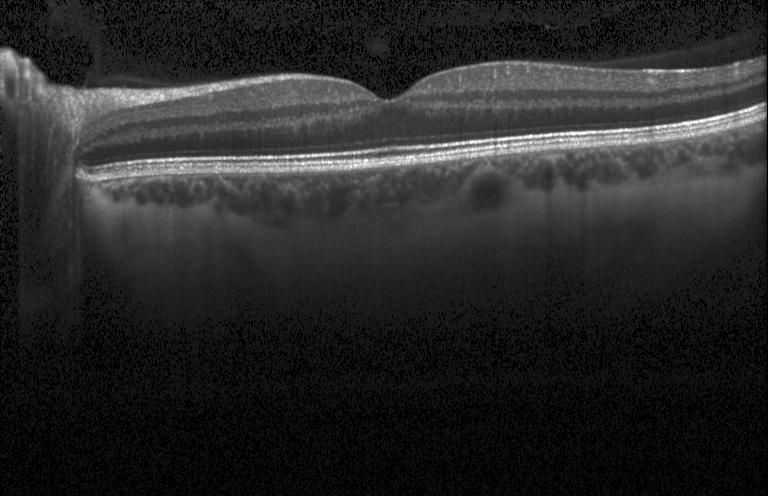 The scan shows no choroidal neovascularization, no diabetic macular edema, and no drusen.